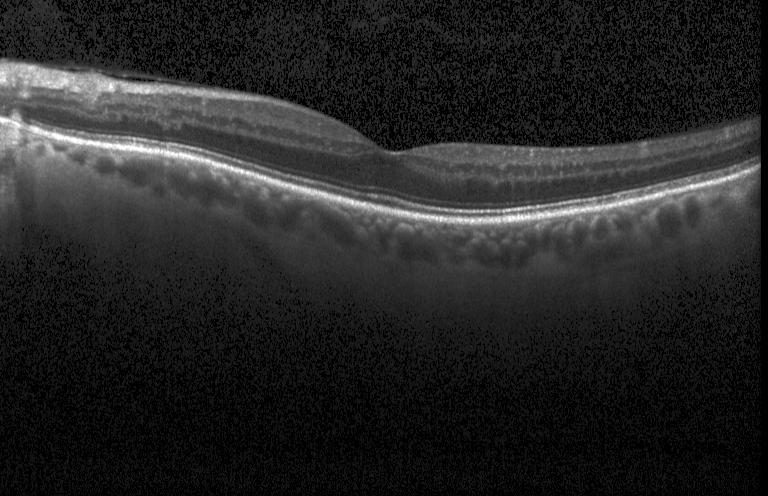
Retinal OCT B-scan, spectral-domain OCT, acquired on a Heidelberg Spectralis. Assessment: no choroidal neovascularization, diabetic macular edema, or drusen.